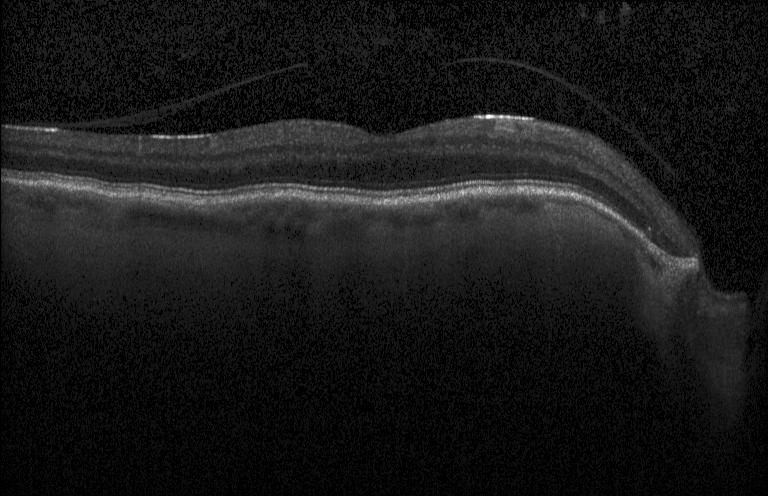
This B-scan demonstrates no CNV, DME, or drusen.